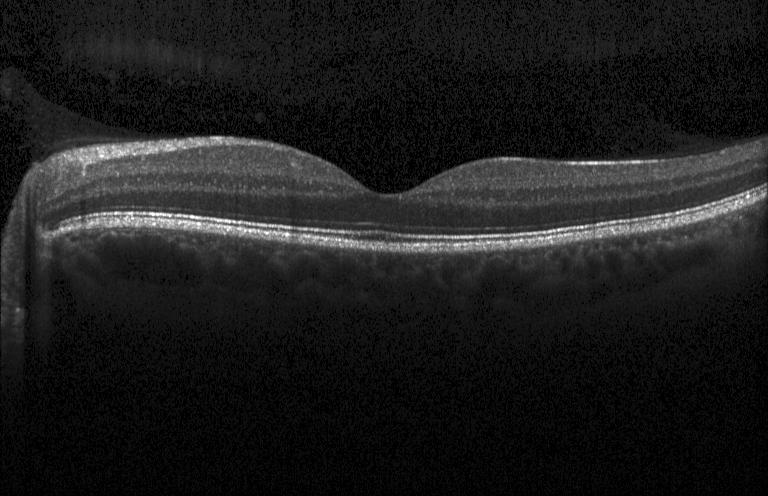 Dx: no evidence of CNV, DME, or drusen.